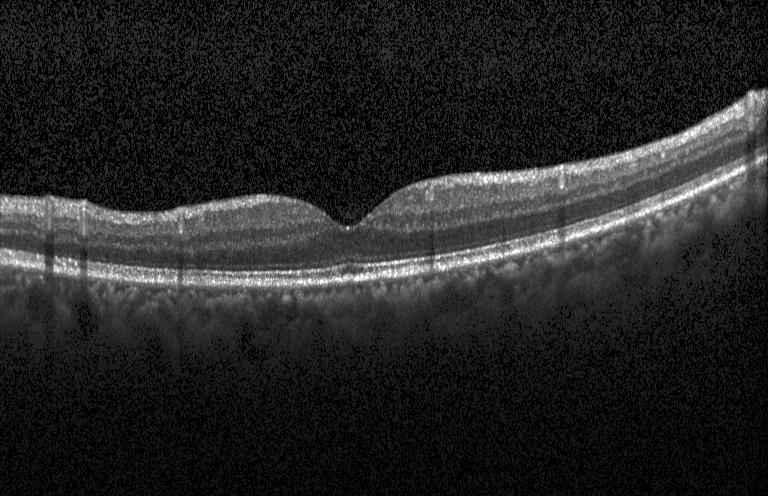
Optical coherence tomography B-scan, Heidelberg Spectralis, spectral-domain optical coherence tomography — The scan shows no choroidal neovascularization, no diabetic macular edema, and no drusen.